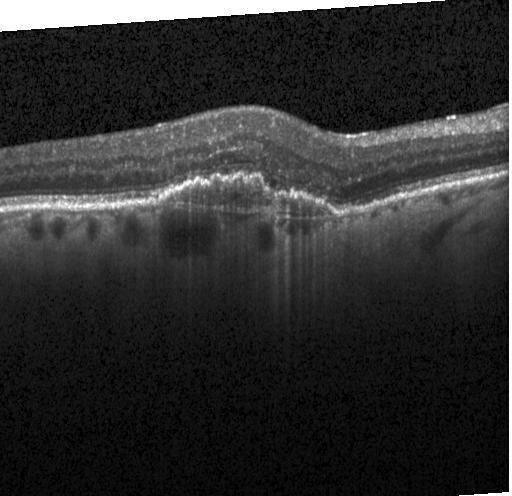 OCT scan showing a choroidal neovascular membrane.